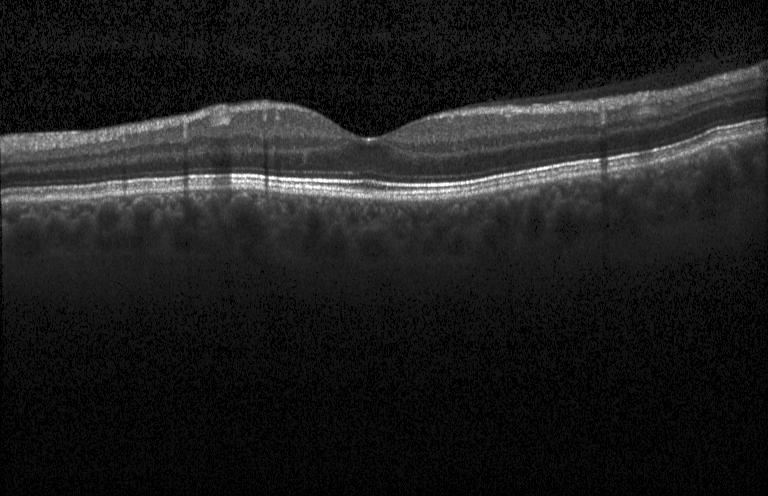
Assessment: no choroidal neovascularization, diabetic macular edema, or drusen.